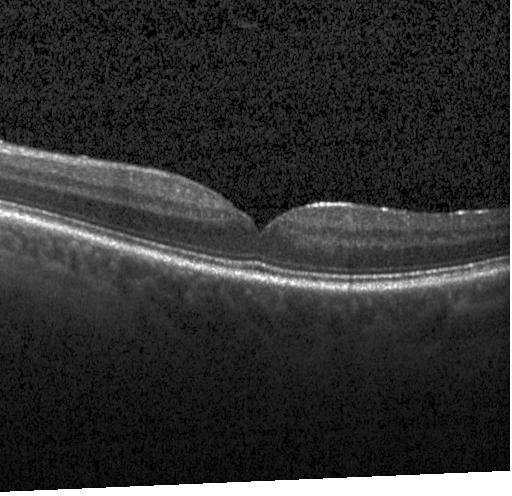

OCT line scan; fovea-centered
This B-scan demonstrates no CNV, no DME, and no drusen.